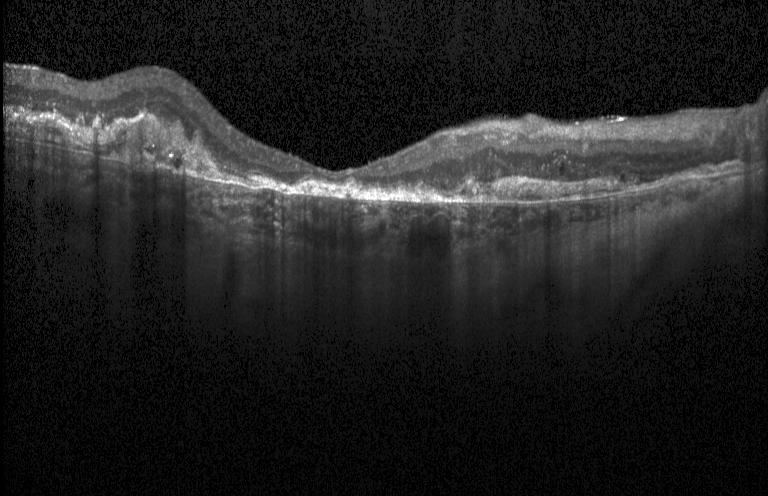
Horizontal scan through the fovea; spectral-domain optical coherence tomography; retinal OCT B-scan.
Choroidal neovascularization.